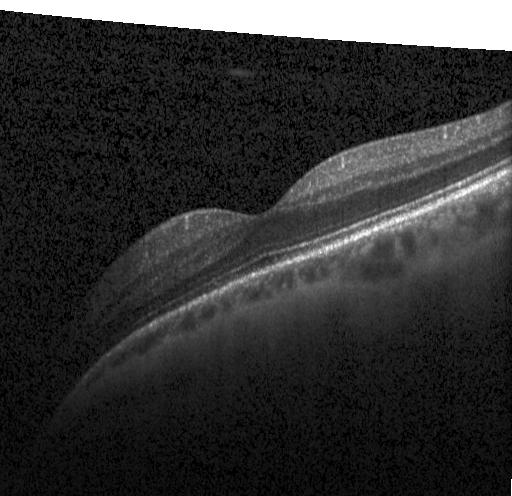 OCT line scan. No evidence of CNV, DME, or drusen.